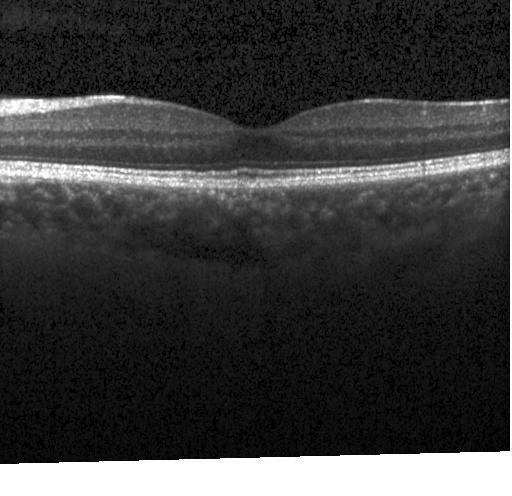
Macular OCT: no CNV, no DME, and no drusen.